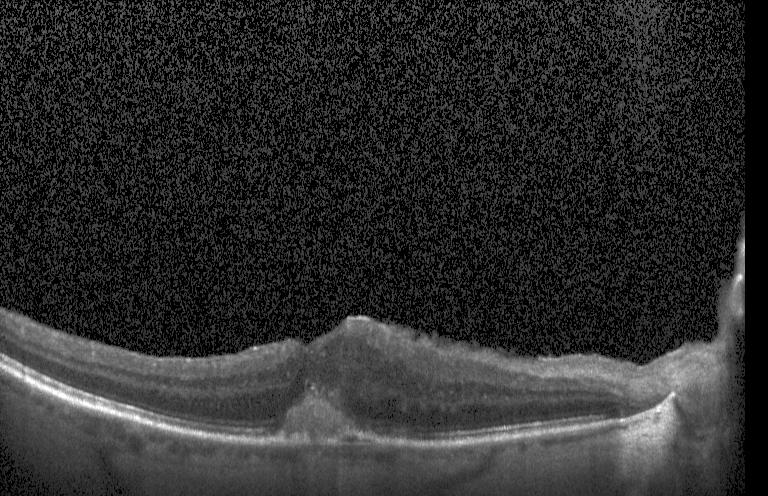

Optical coherence tomography scan. Instrument: Heidelberg Spectralis. Fovea-centered
OCT finding: a choroidal neovascular membrane.